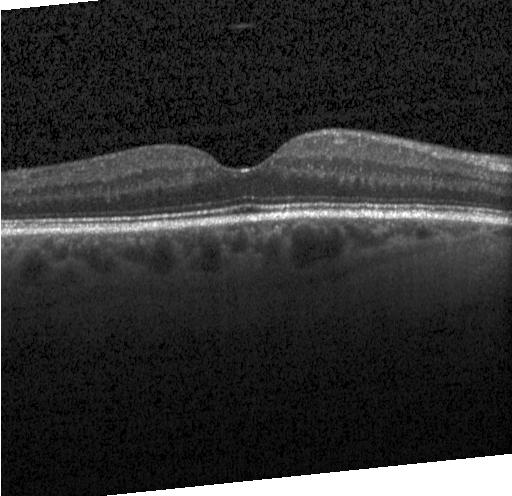 SD-OCT · through the macula · retinal OCT B-scan · acquired on a Heidelberg Spectralis.
Diagnosis: neither choroidal neovascularization, diabetic macular edema, nor drusen.